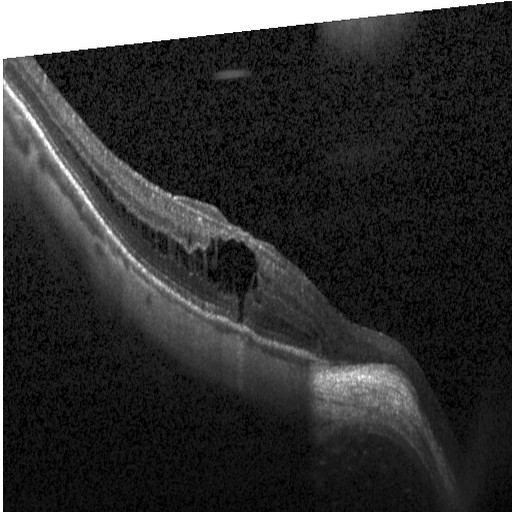
Retinal OCT cross-section showing DME.